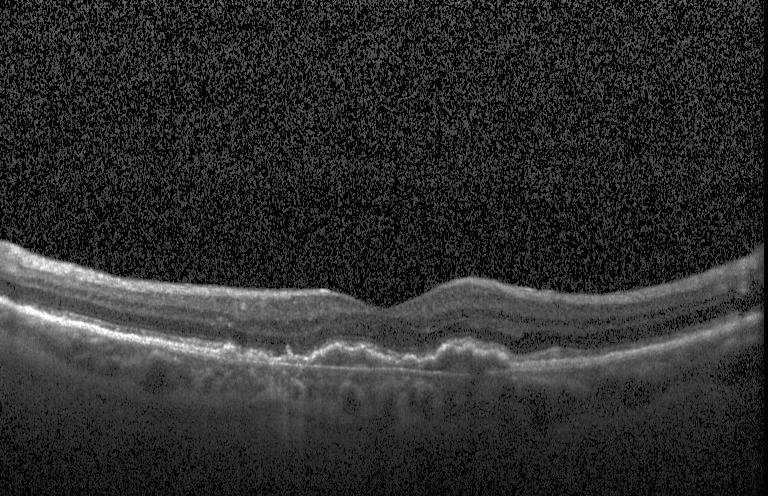

Spectral-domain OCT; horizontal scan through the fovea; OCT B-scan
Assessment: a choroidal neovascular membrane.